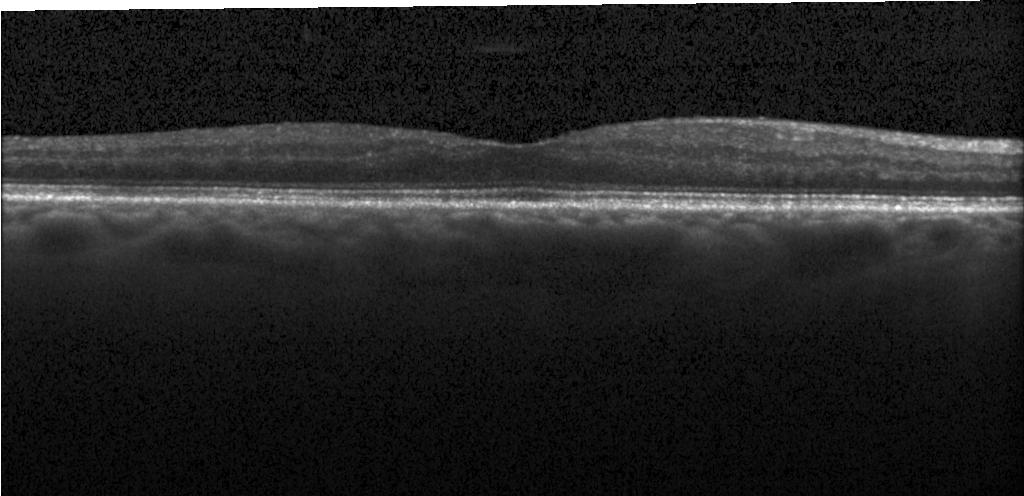

Instrument: Heidelberg Spectralis; retinal OCT B-scan; spectral-domain OCT. Impression: no evidence of choroidal neovascularization, diabetic macular edema, or drusen.